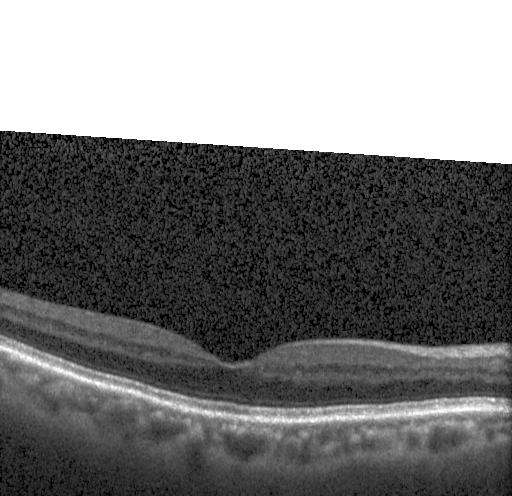
Dx: no evidence of choroidal neovascularization, diabetic macular edema, or drusen.